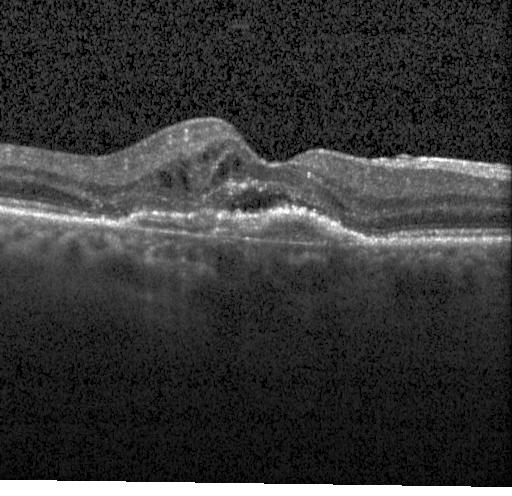

Macular OCT: a choroidal neovascular membrane.